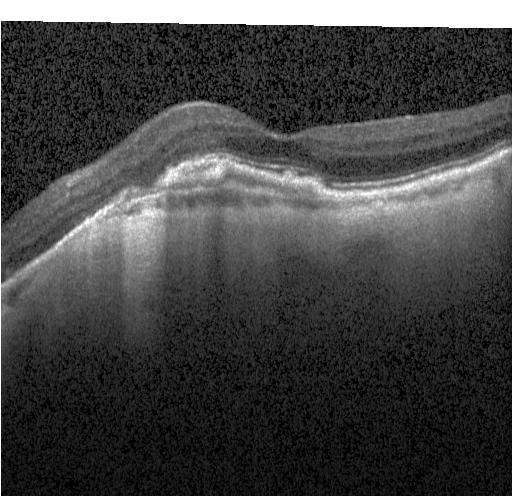

Macular OCT: a choroidal neovascular membrane.